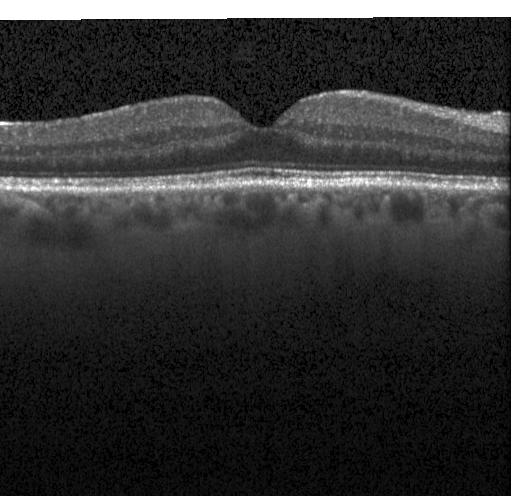

Heidelberg Spectralis, horizontal scan through the fovea, retinal OCT B-scan, SD-OCT. No choroidal neovascularization, no diabetic macular edema, and no drusen.